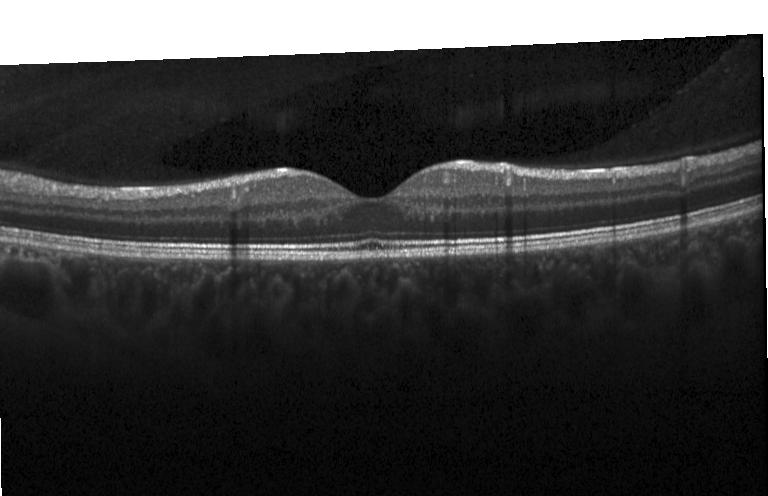
Finding: no choroidal neovascularization, diabetic macular edema, or drusen.